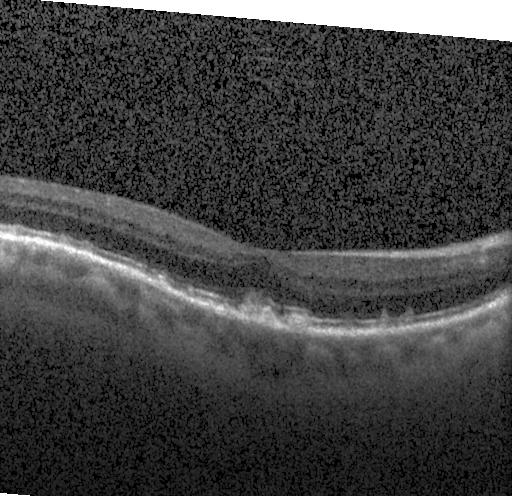
OCT B-scan; instrument: Heidelberg Spectralis — Assessment: multiple drusen.